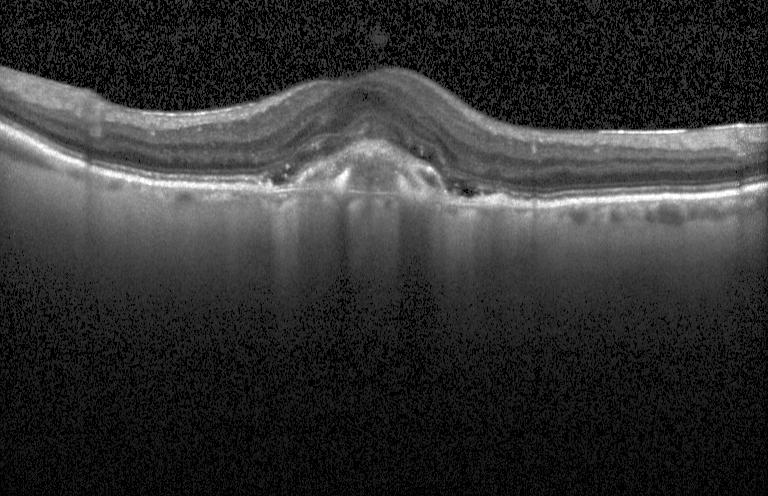

Spectral-domain OCT B-scan: a choroidal neovascular membrane.